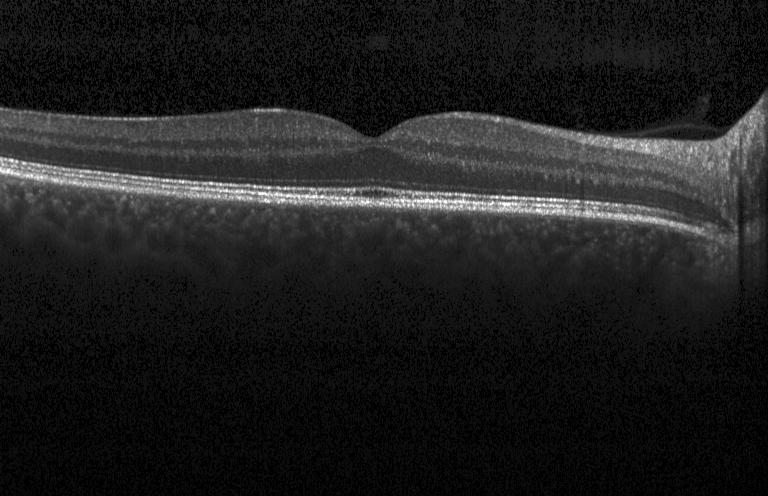 Finding: neither CNV, DME, nor drusen.